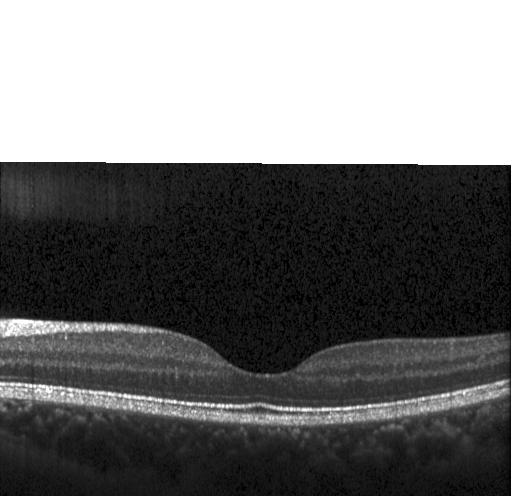

Heidelberg Spectralis, through the macula, OCT B-scan, SD-OCT — Macular OCT: no CNV, no DME, and no drusen.